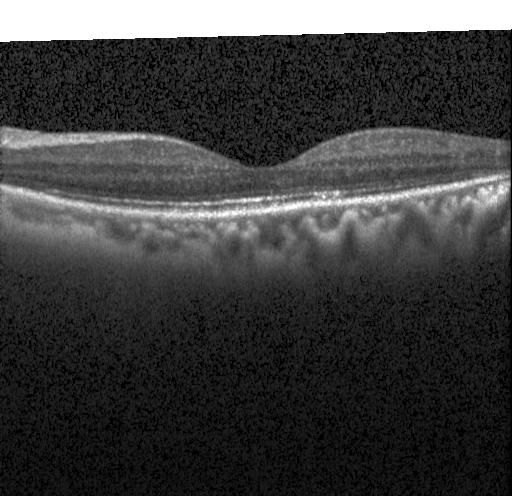
Finding: neither choroidal neovascularization, diabetic macular edema, nor drusen.